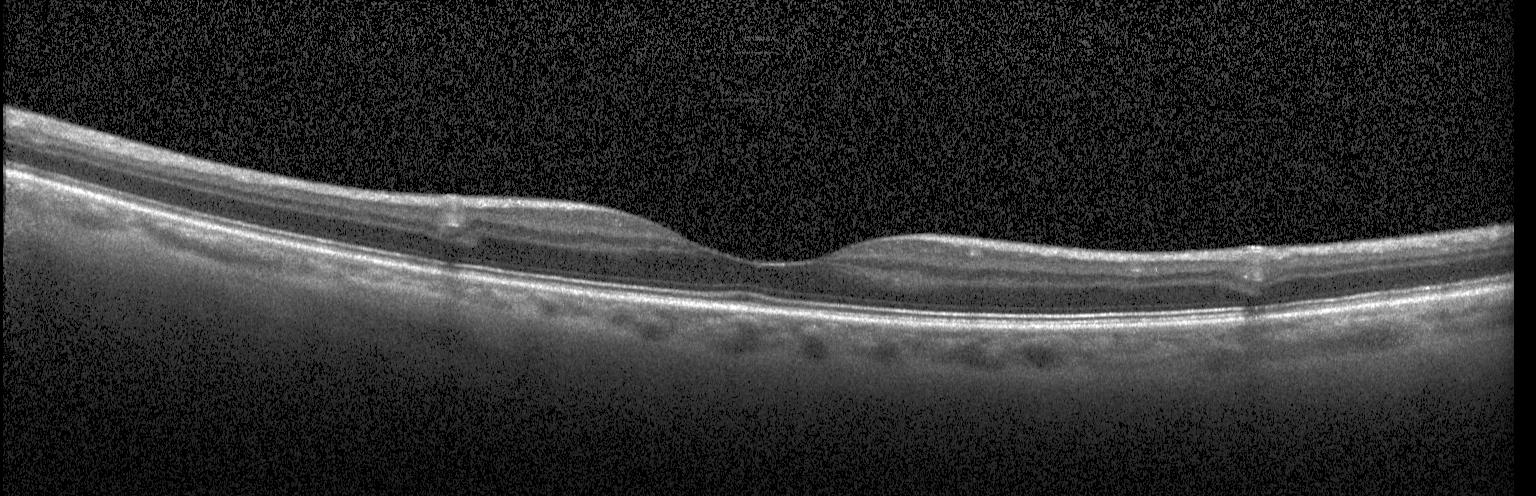 Optical coherence tomography scan.
Diagnosis: no choroidal neovascularization, diabetic macular edema, or drusen.